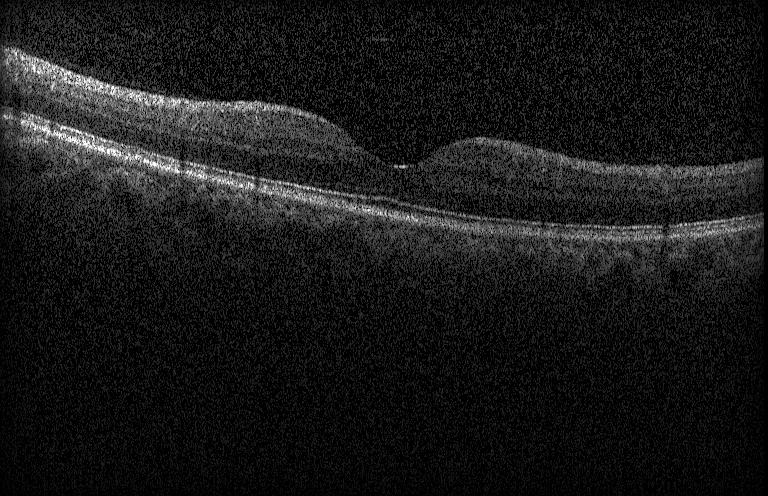 OCT B-scan showing no choroidal neovascularization, no diabetic macular edema, and no drusen.